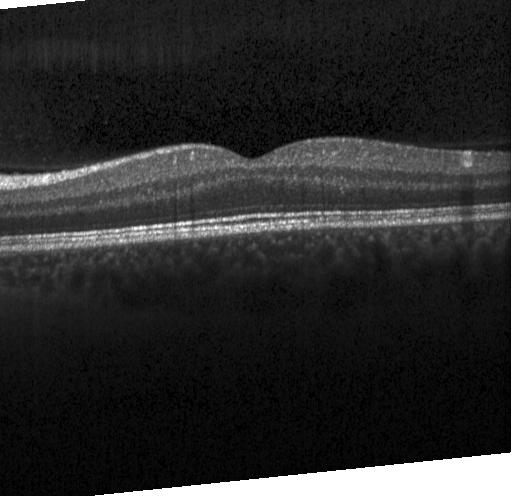
Spectral-domain OCT · OCT line scan.
Assessment: no evidence of CNV, DME, or drusen.